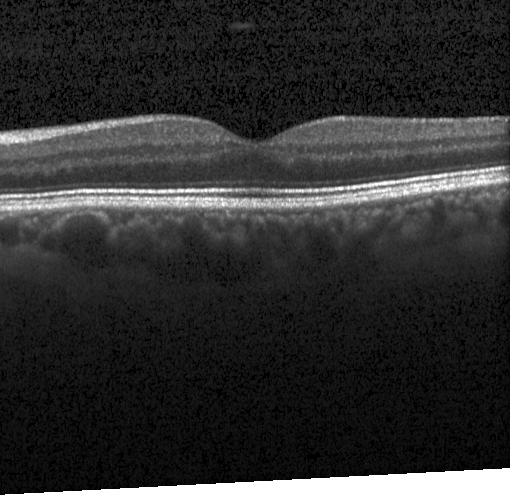 OCT line scan — Impression: no choroidal neovascularization, diabetic macular edema, or drusen.